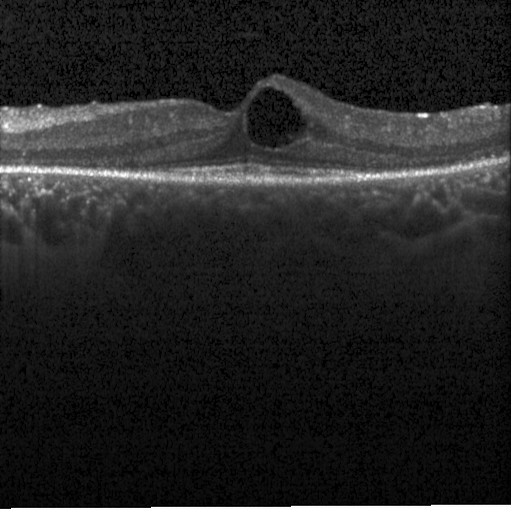

Retinal OCT B-scan; fovea-centered — The scan shows diabetic macular edema (DME).